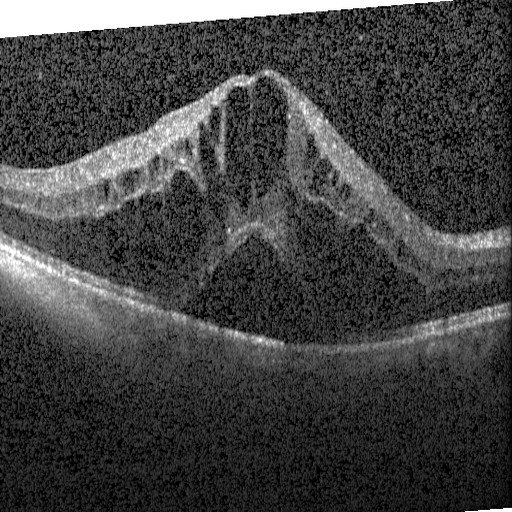
Macular OCT: diabetic macular edema (DME).